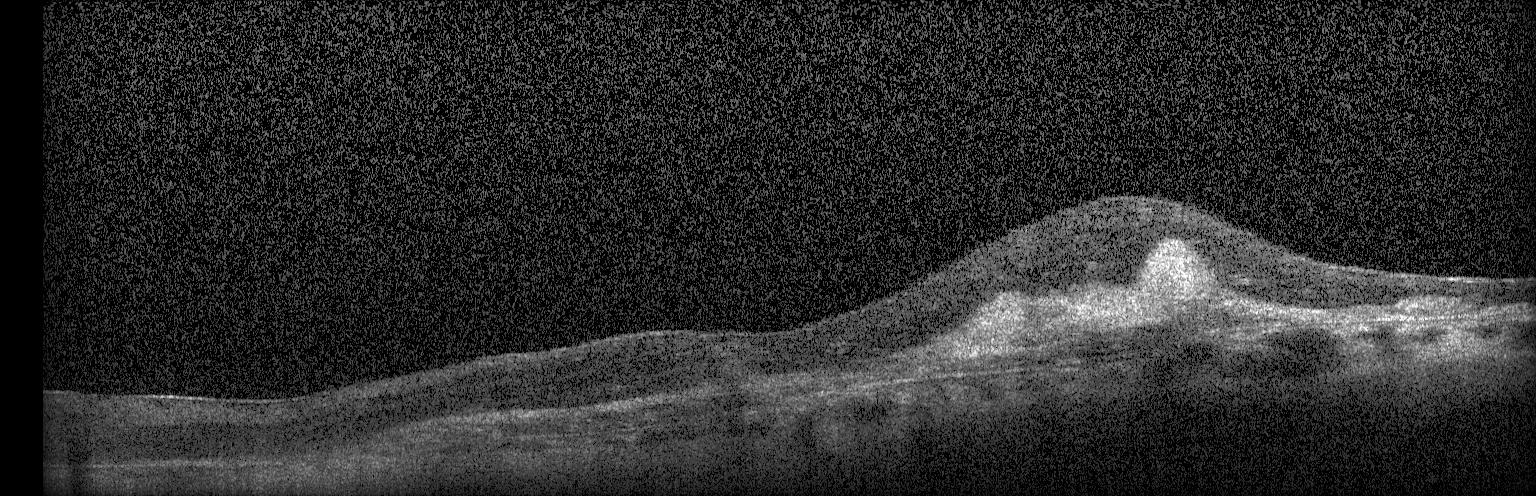 Optical coherence tomography B-scan, SD-OCT, through the macula. The scan shows a choroidal neovascular membrane.